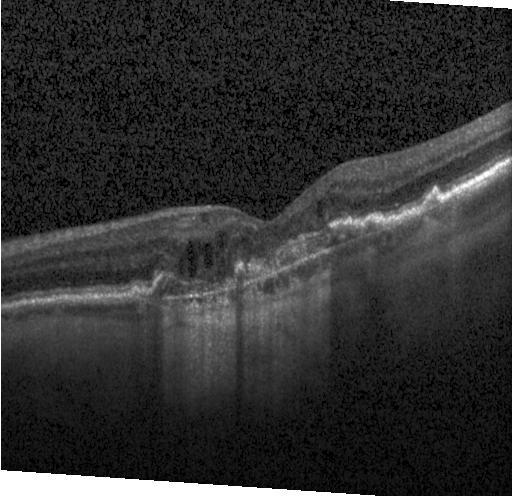

Retinal OCT cross-section — The scan shows a choroidal neovascular membrane.